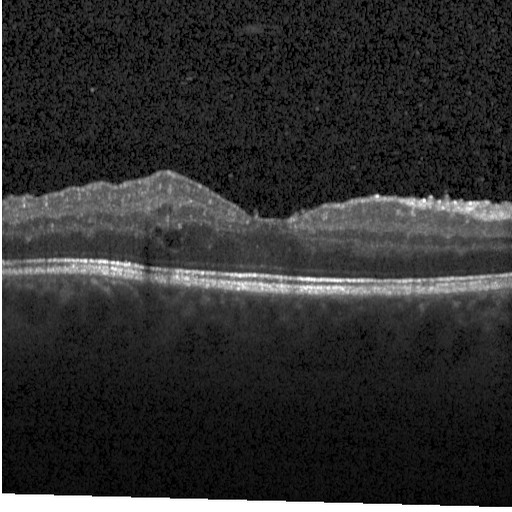 Centered on the fovea. Optical coherence tomography B-scan. Instrument: Heidelberg Spectralis
Impression: diabetic macular edema (DME).